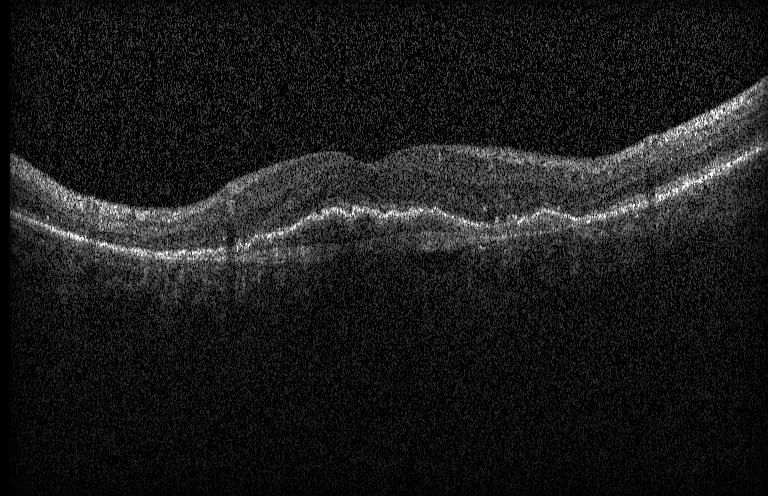
Assessment: a choroidal neovascular membrane.